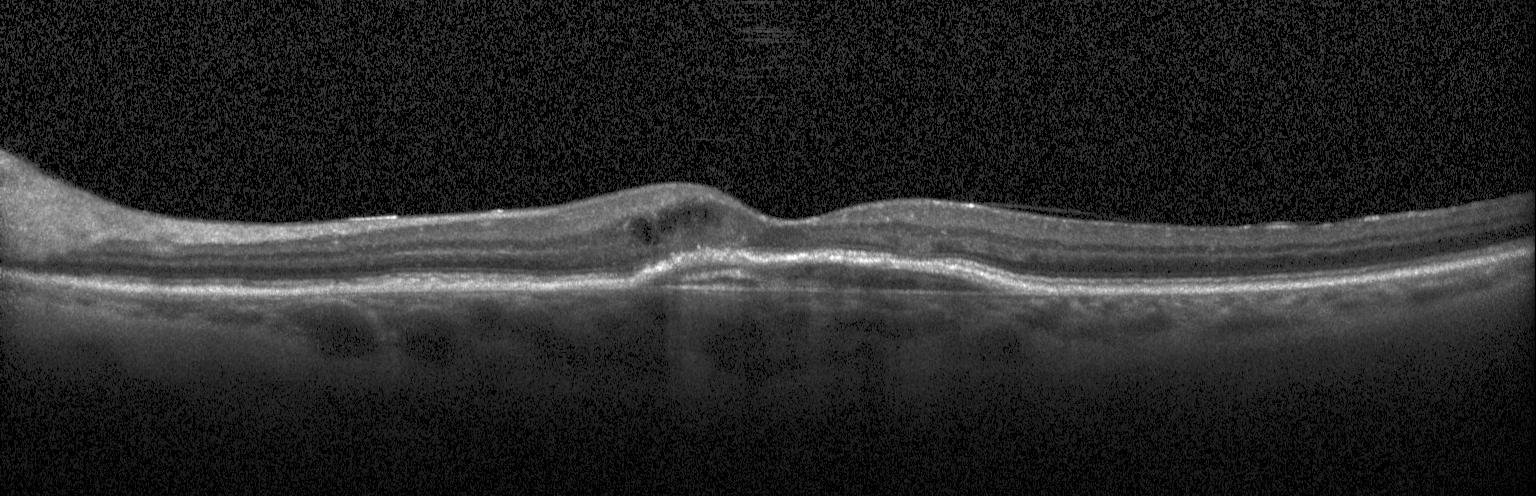 Spectral-domain OCT, retinal OCT B-scan, Heidelberg Spectralis OCT system. The scan shows choroidal neovascularization (CNV).